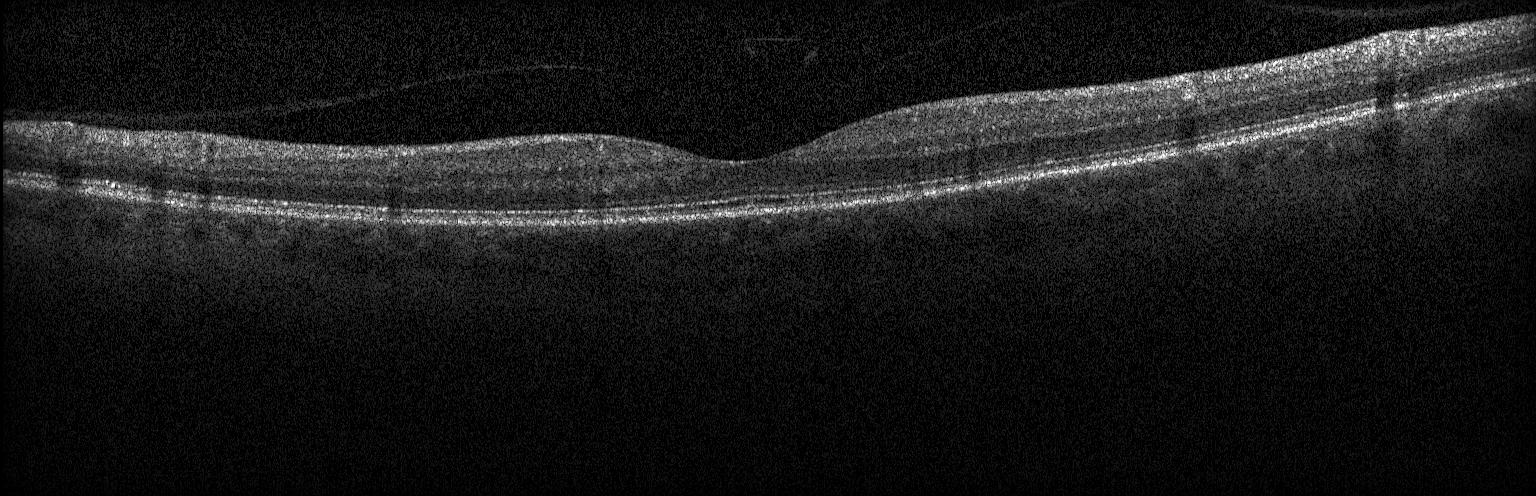
Instrument: Heidelberg Spectralis. OCT B-scan
Finding: no evidence of CNV, DME, or drusen.